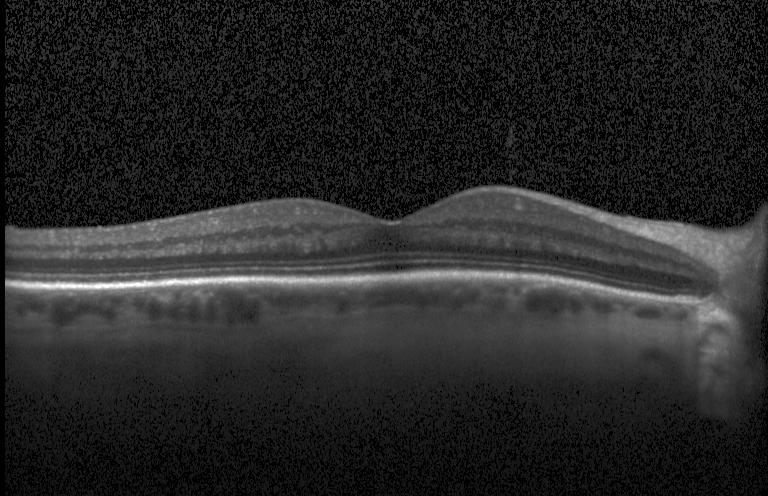

OCT B-scan showing no CNV, DME, or drusen.